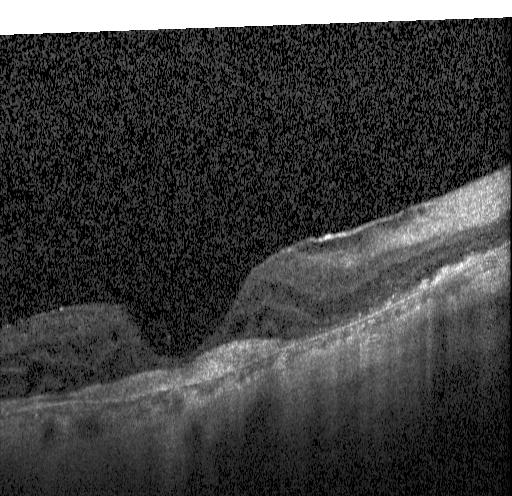 Heidelberg Spectralis OCT system · retinal OCT cross-section · horizontal scan through the fovea. Impression: choroidal neovascularization.